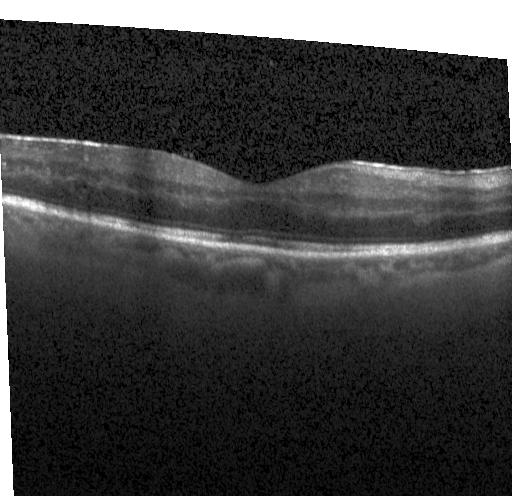 Impression: no choroidal neovascularization, no diabetic macular edema, and no drusen.